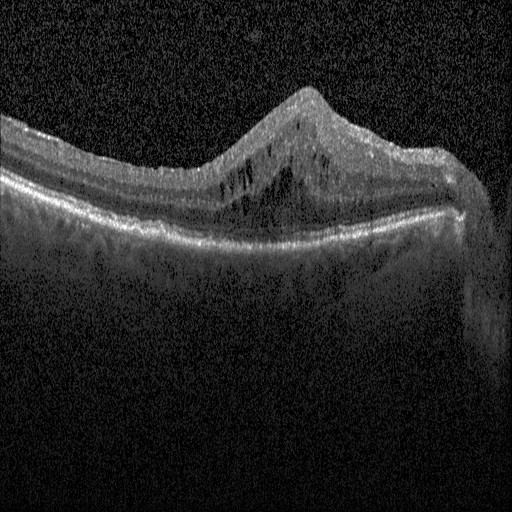 Diabetic macular edema.